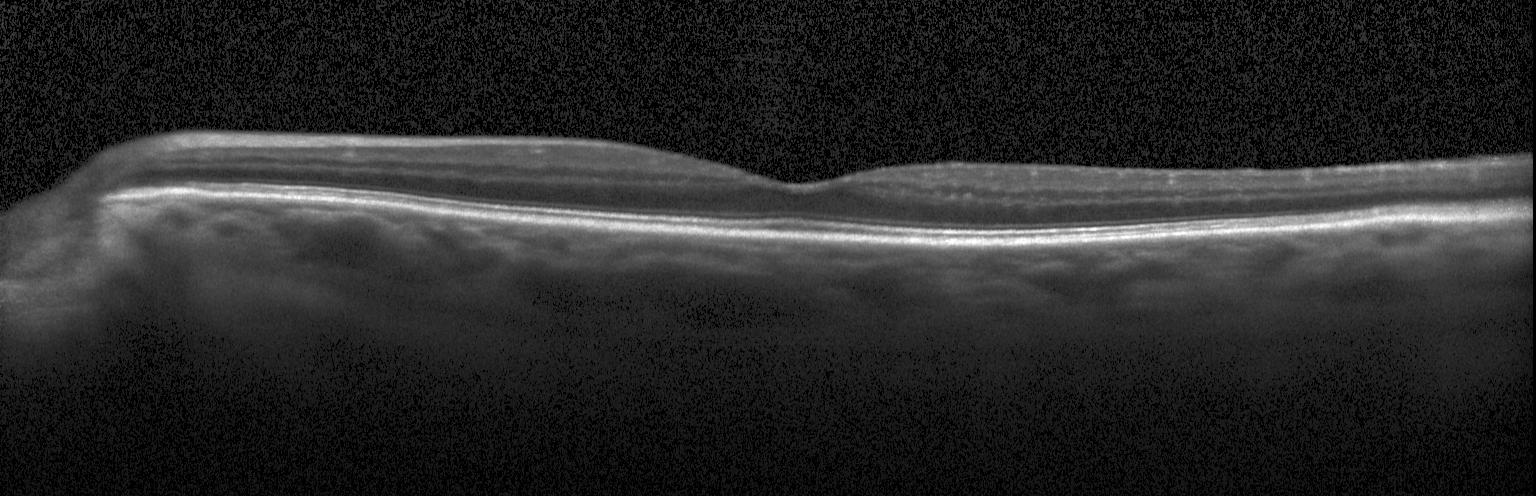
No choroidal neovascularization, diabetic macular edema, or drusen.